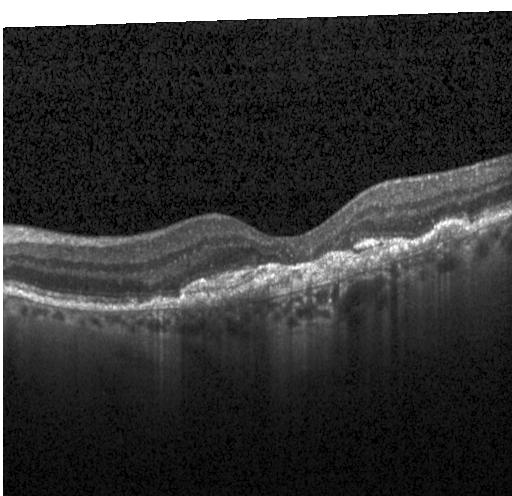
Spectral-domain optical coherence tomography; instrument: Heidelberg Spectralis; optical coherence tomography B-scan — Impression: CNV.